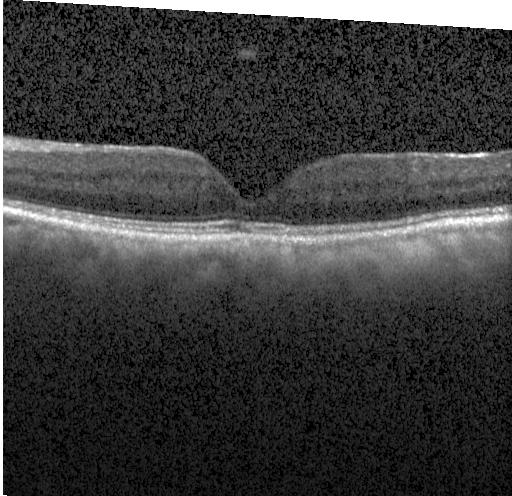 Assessment: neither CNV, DME, nor drusen.